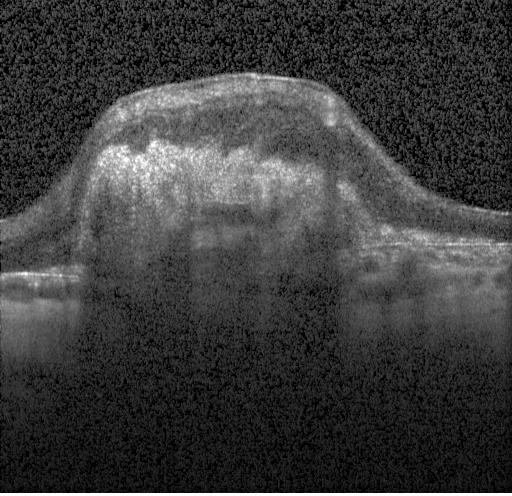
Through the macula; spectral-domain OCT; acquired on a Heidelberg Spectralis; OCT B-scan
The scan shows a choroidal neovascular membrane.